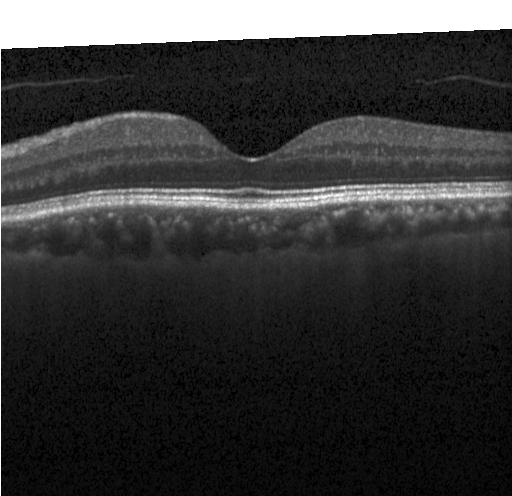 Macular OCT: neither choroidal neovascularization, diabetic macular edema, nor drusen.